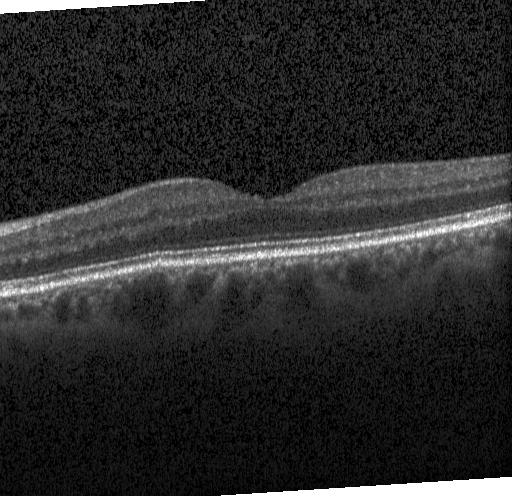 Assessment: no evidence of choroidal neovascularization, diabetic macular edema, or drusen.